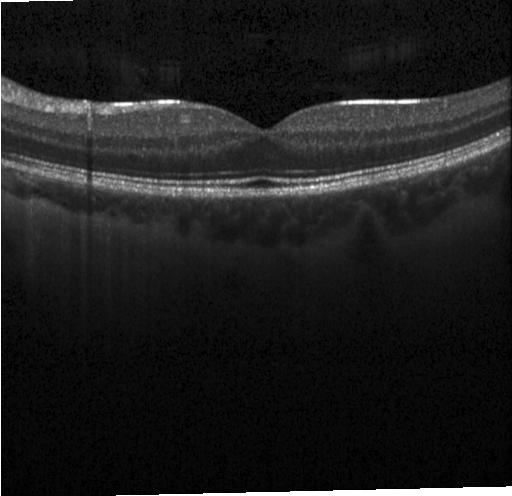

Horizontal scan through the fovea, spectral-domain optical coherence tomography, retinal OCT cross-section, Heidelberg Spectralis.
Impression: no CNV, DME, or drusen.